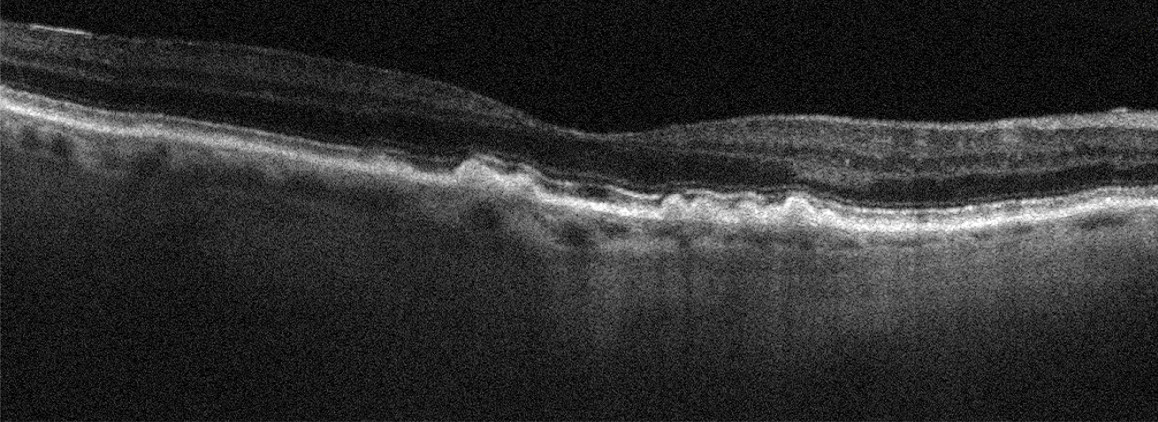 Optical coherence tomography scan — Age-related macular degeneration.